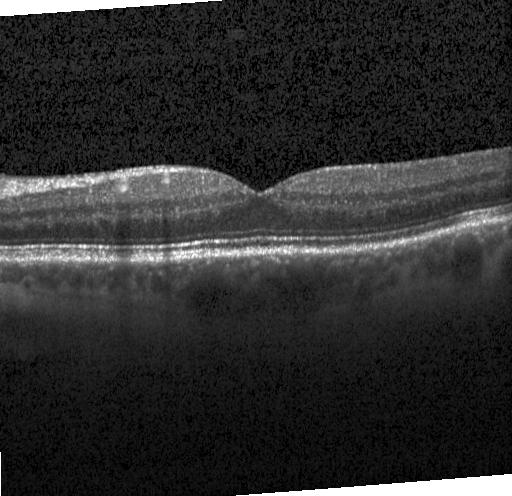

OCT line scan; macular scan — Finding: no choroidal neovascularization, no diabetic macular edema, and no drusen.